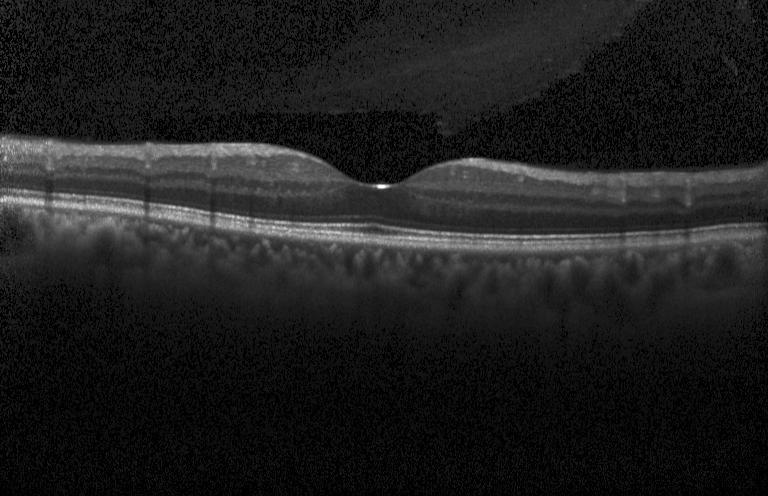
Retinal OCT cross-section showing no evidence of CNV, DME, or drusen.